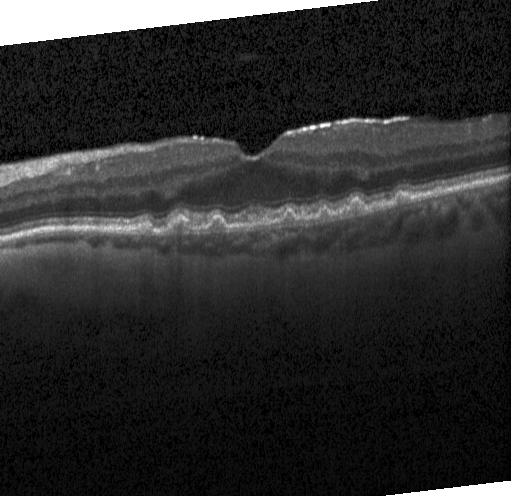 Instrument: Heidelberg Spectralis, OCT line scan, spectral-domain OCT, centered on the fovea
Diagnosis: drusen.